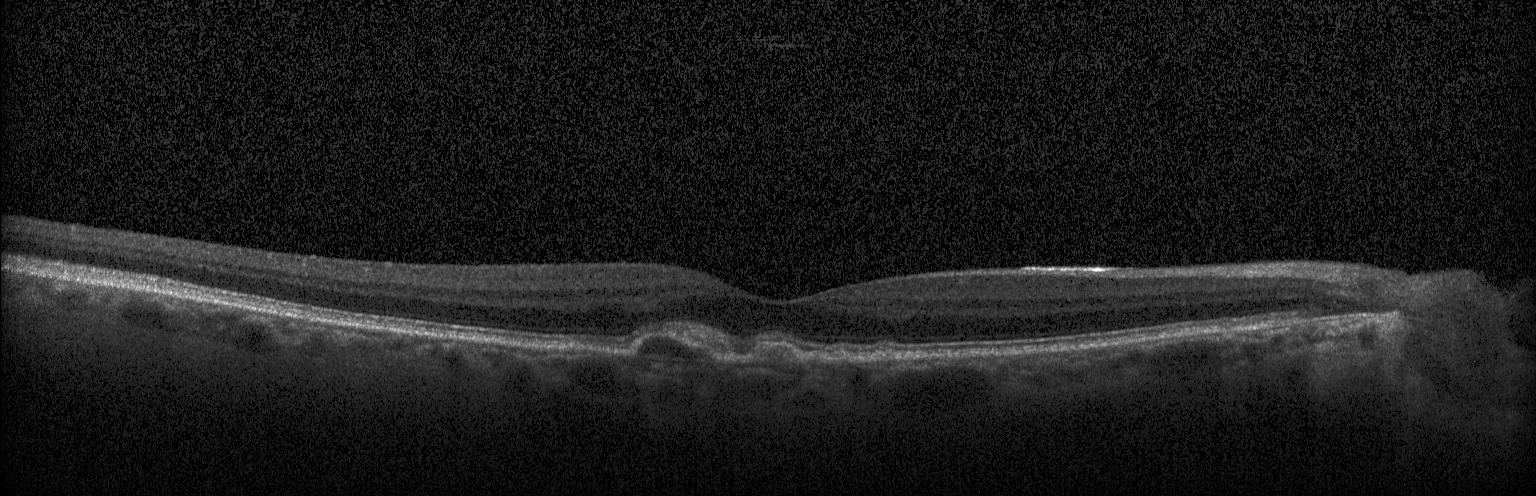

Macular OCT demonstrating a choroidal neovascular membrane.